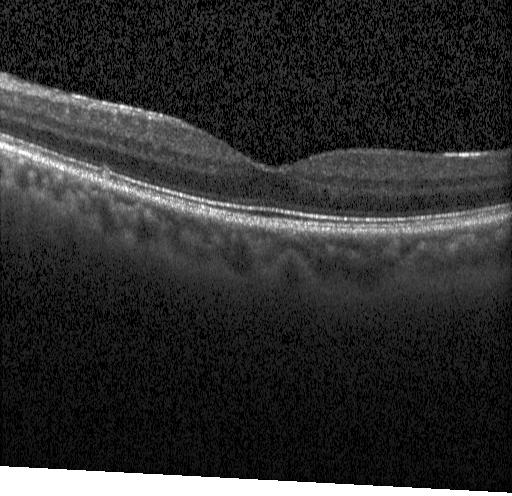

SD-OCT. OCT line scan. Fovea-centered. Instrument: Heidelberg Spectralis.
OCT finding: no evidence of choroidal neovascularization, diabetic macular edema, or drusen.